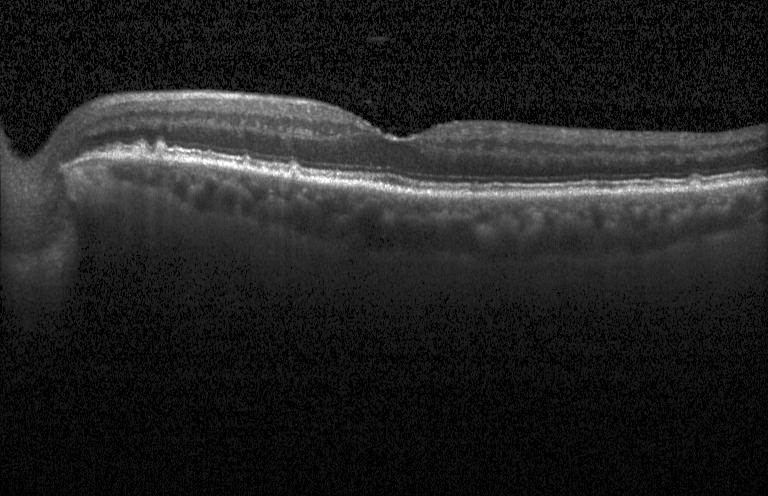
Acquired on a Heidelberg Spectralis; OCT line scan
The scan shows drusen.